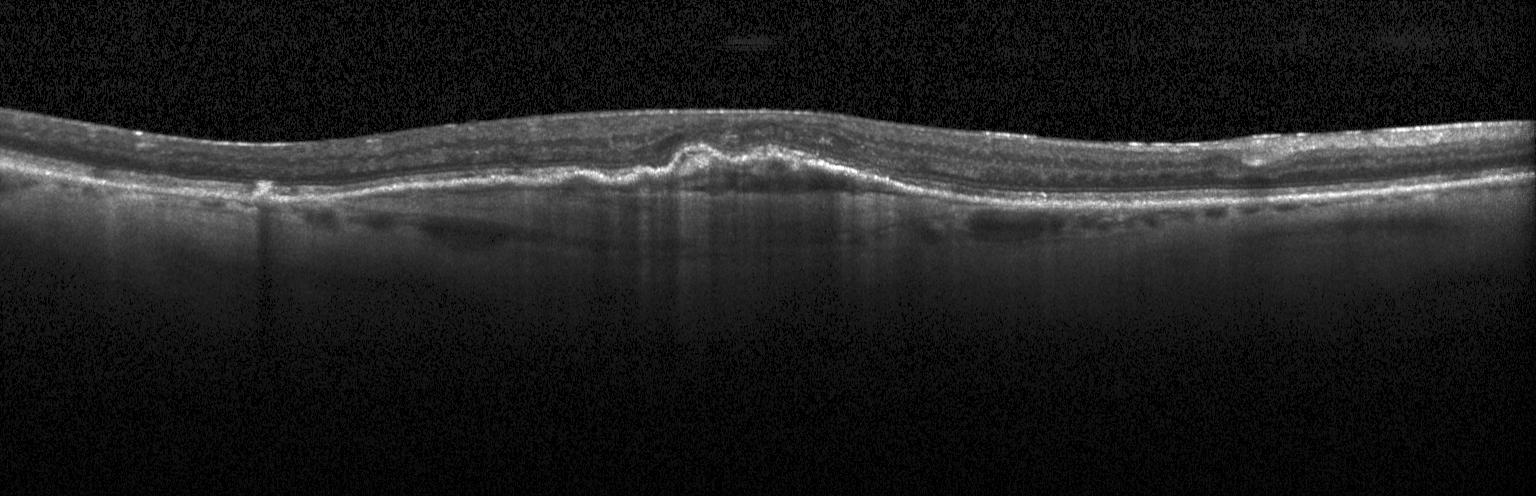

OCT B-scan. Spectral-domain OCT
Macular OCT: a choroidal neovascular membrane.